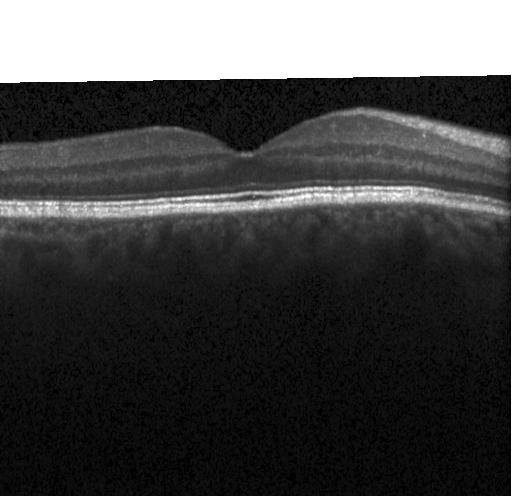 Retinal OCT cross-section; Heidelberg Spectralis OCT system; horizontal scan through the fovea; spectral-domain optical coherence tomography
Finding: no choroidal neovascularization, no diabetic macular edema, and no drusen.